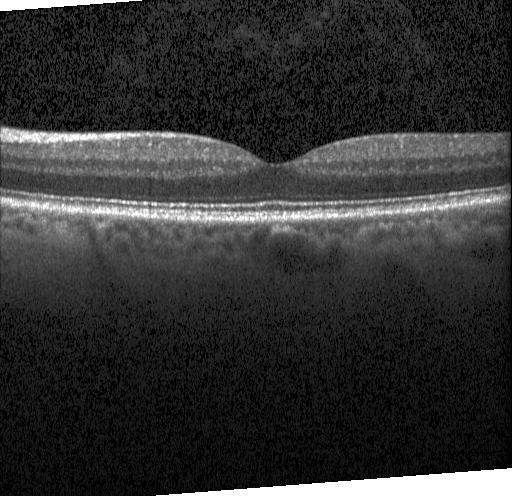

Retinal OCT B-scan. Assessment: no evidence of choroidal neovascularization, diabetic macular edema, or drusen.